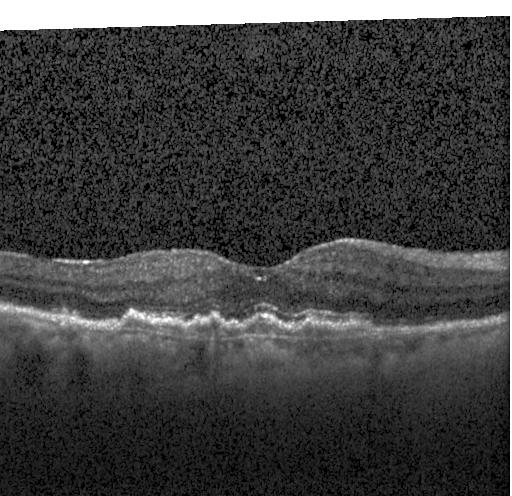

Optical coherence tomography scan. Dx: CNV.